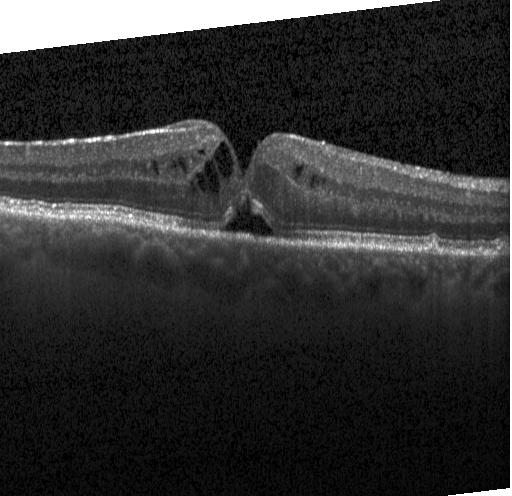

Retinal OCT cross-section.
The scan shows DME.